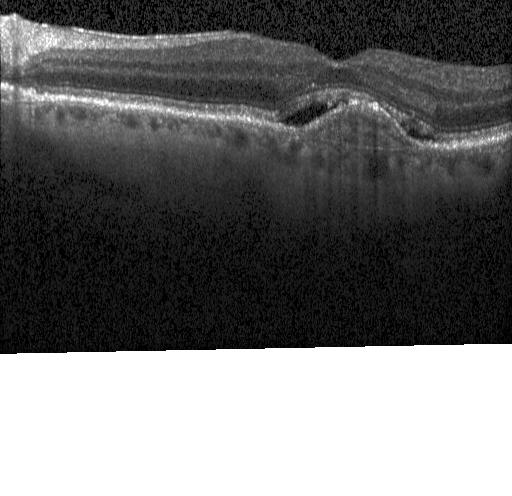
Finding: choroidal neovascularization.